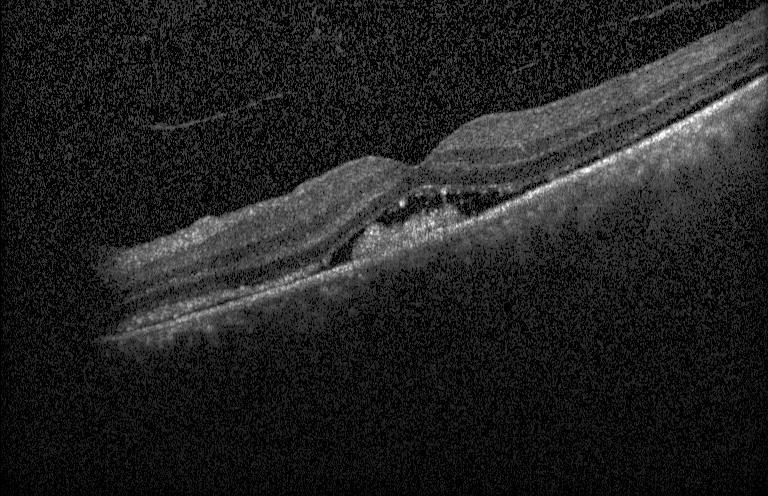

OCT line scan, macular scan, Heidelberg Spectralis.
Macular OCT: choroidal neovascularization.